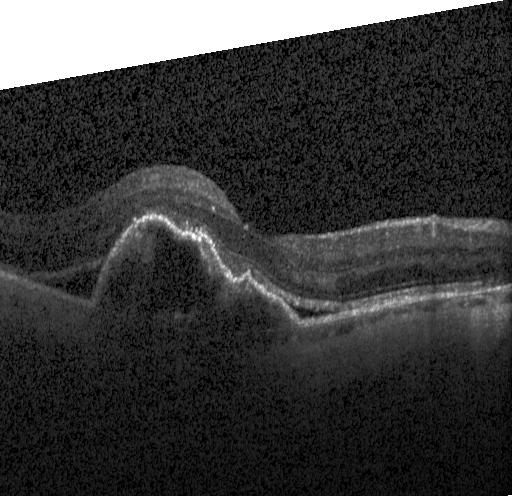
Optical coherence tomography scan
The scan shows a choroidal neovascular membrane.